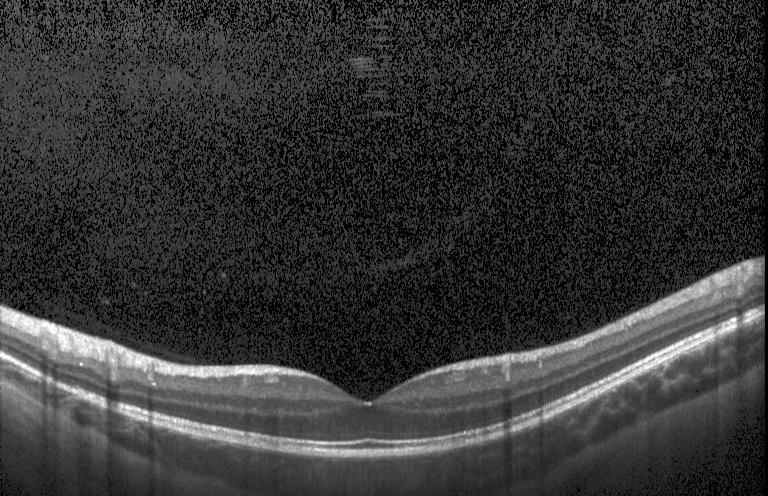 Spectral-domain optical coherence tomography, retinal OCT B-scan — Finding: neither choroidal neovascularization, diabetic macular edema, nor drusen.